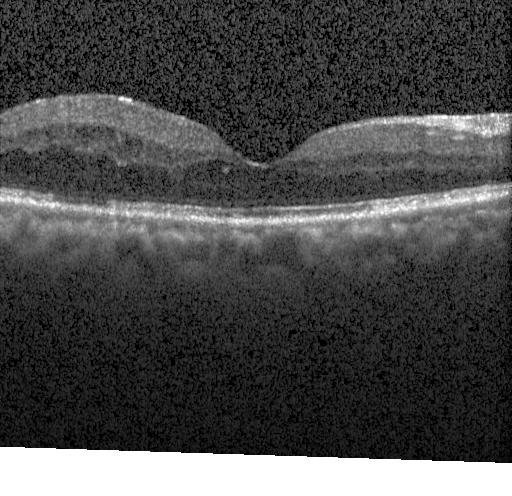
Macular scan · retinal OCT cross-section — Finding: diabetic macular edema (DME).